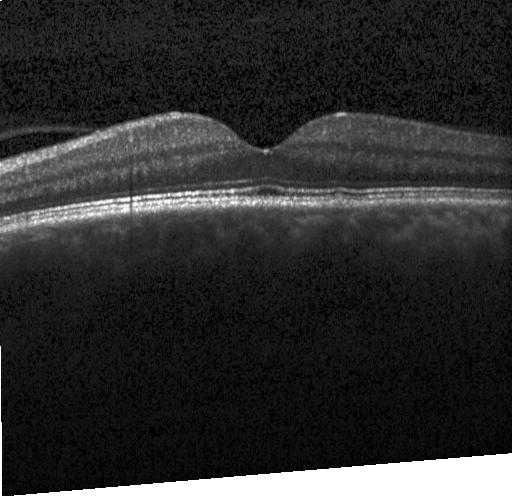

Finding: no choroidal neovascularization, diabetic macular edema, or drusen.